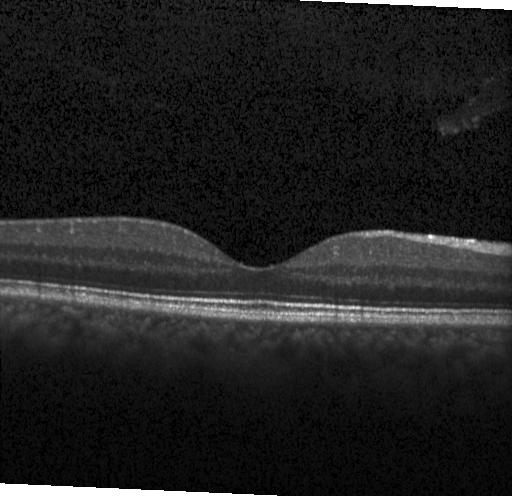 Spectral-domain optical coherence tomography; acquired on a Heidelberg Spectralis; macular scan; retinal OCT cross-section
OCT finding: no evidence of choroidal neovascularization, diabetic macular edema, or drusen.